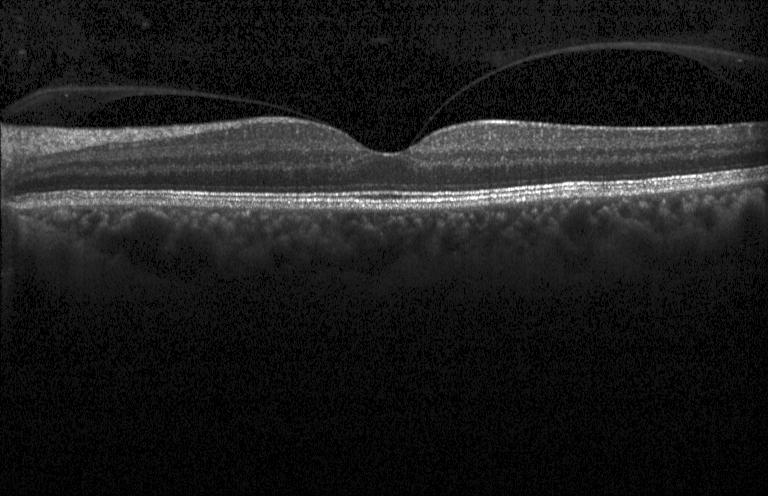
Instrument: Heidelberg Spectralis · OCT line scan. Macular OCT: neither CNV, DME, nor drusen.